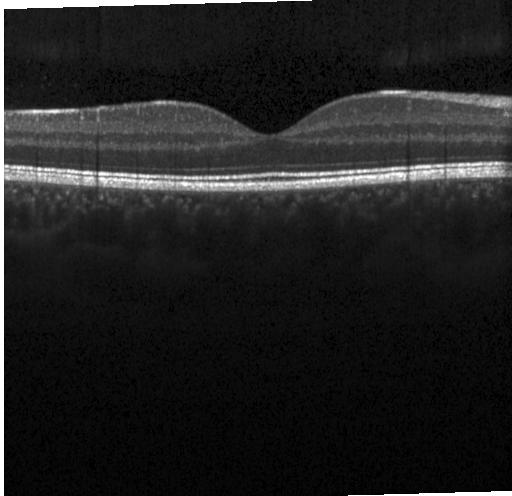
Optical coherence tomography B-scan; macular scan; spectral-domain optical coherence tomography; Heidelberg Spectralis OCT system — Macular OCT: no choroidal neovascularization, diabetic macular edema, or drusen.